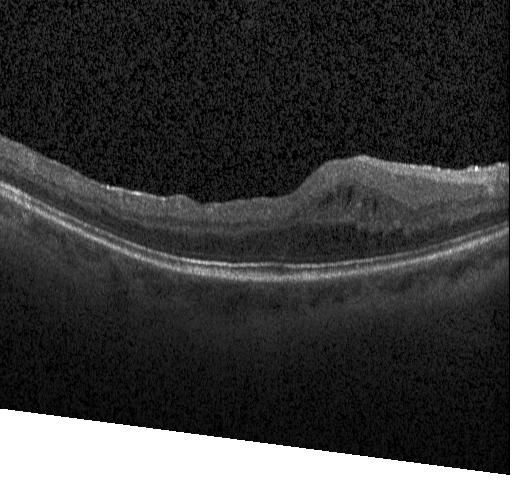 Diabetic macular edema.